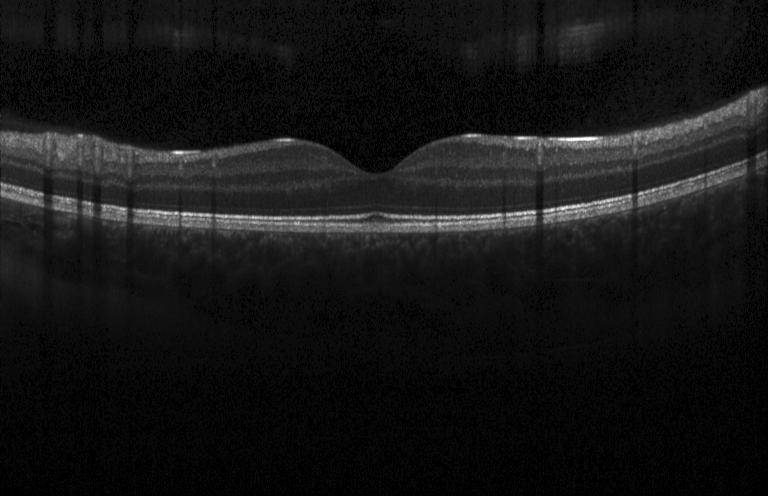 OCT B-scan. SD-OCT. Macular scan. Heidelberg Spectralis OCT system — Diagnosis: neither choroidal neovascularization, diabetic macular edema, nor drusen.